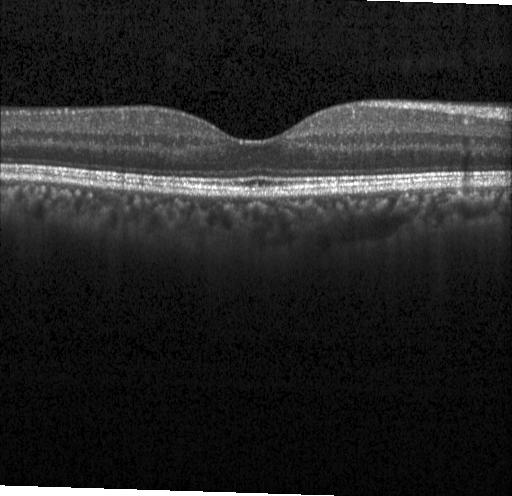
This B-scan demonstrates no CNV, DME, or drusen.